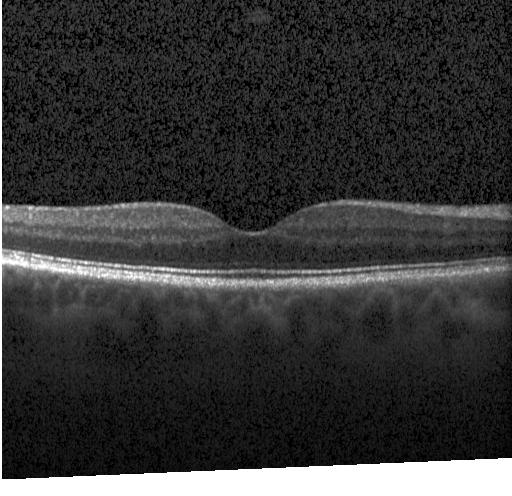
Neither choroidal neovascularization, diabetic macular edema, nor drusen.